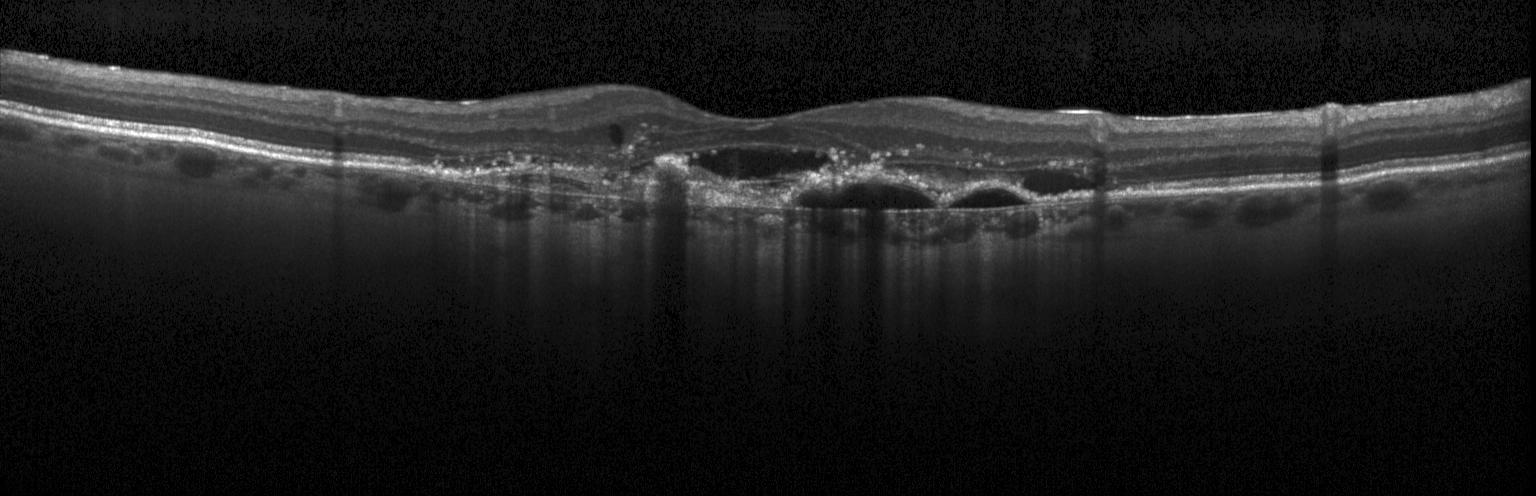

OCT B-scan. Impression: CNV.